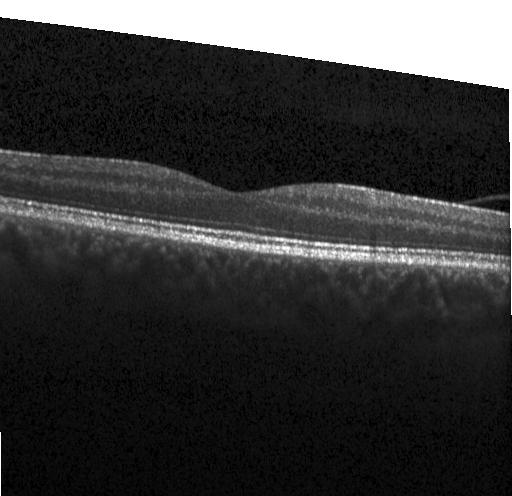
Macular OCT: no choroidal neovascularization, diabetic macular edema, or drusen.